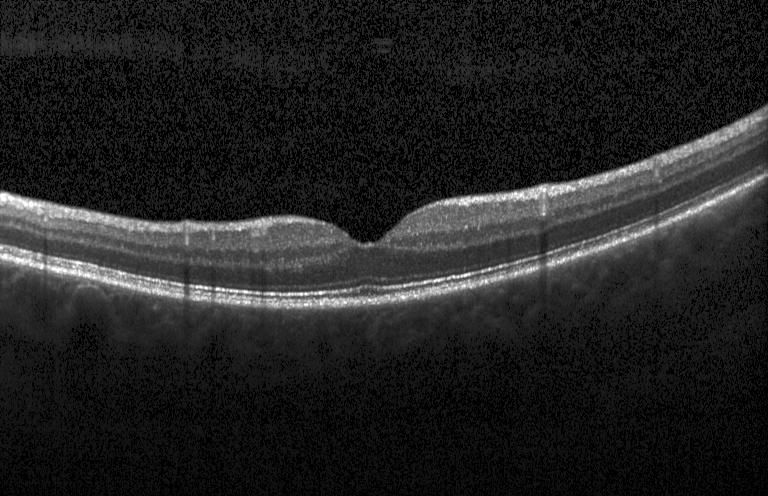
OCT scan showing no evidence of choroidal neovascularization, diabetic macular edema, or drusen.